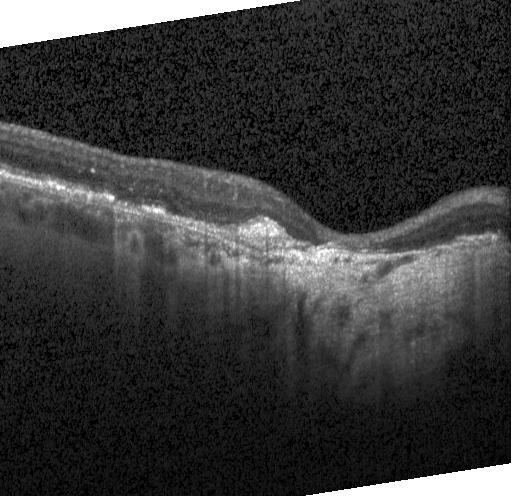

SD-OCT, OCT line scan
Macular OCT: CNV.